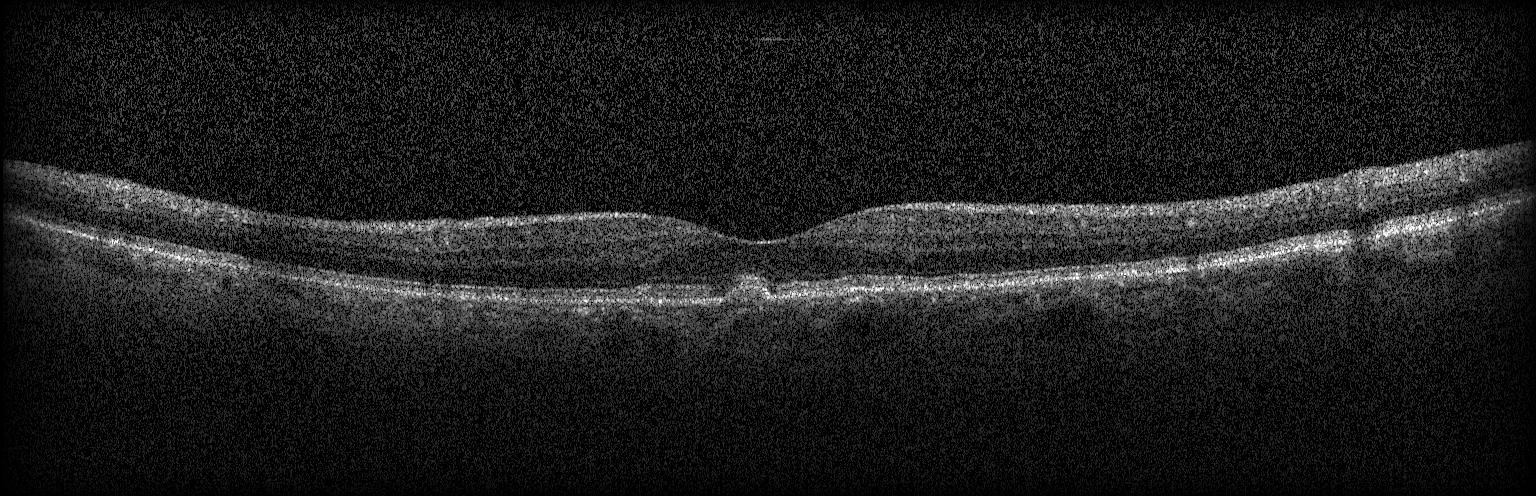
Retinal OCT cross-section showing drusen.